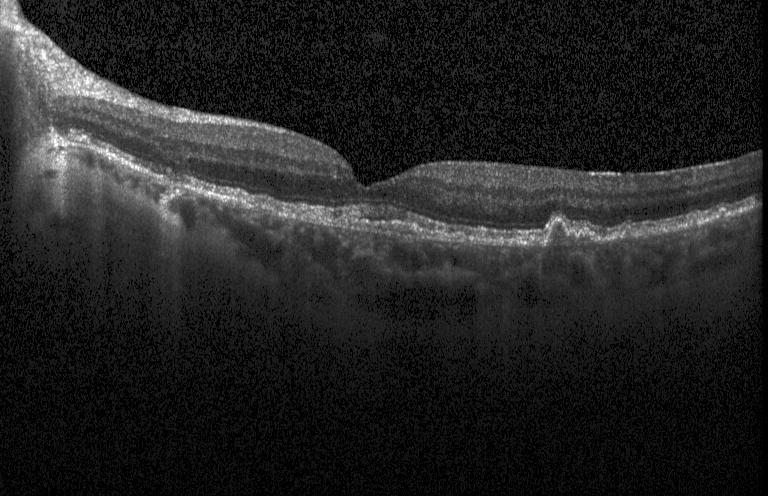

Through the macula; spectral-domain OCT; optical coherence tomography B-scan; Heidelberg Spectralis — Finding: choroidal neovascularization.